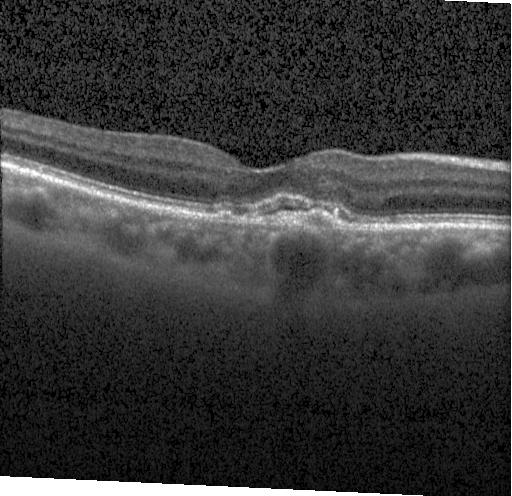

Impression: a choroidal neovascular membrane.